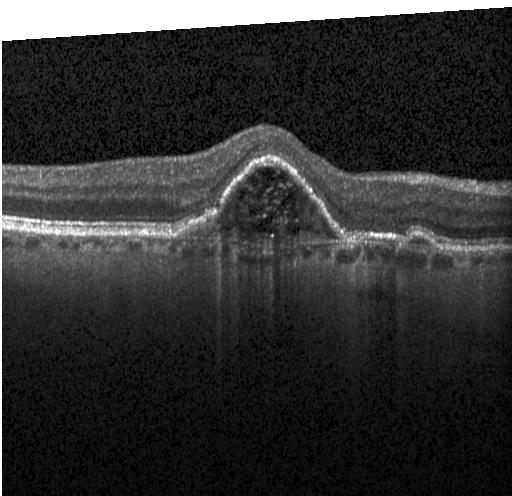 Finding: a choroidal neovascular membrane.